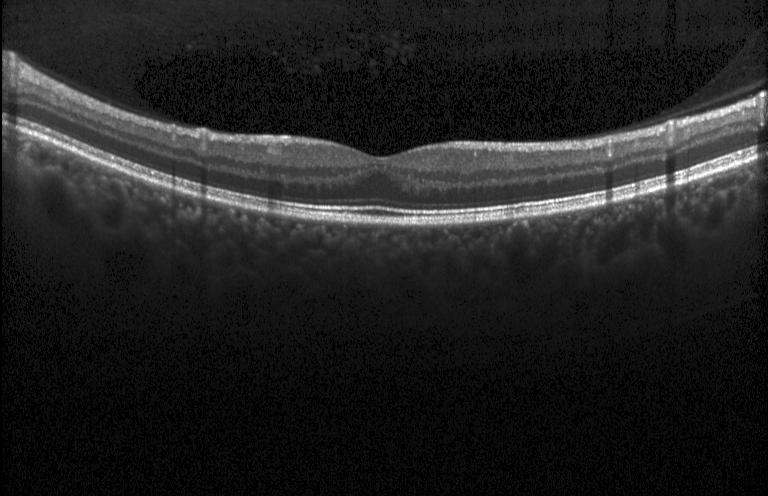

OCT line scan
No evidence of CNV, DME, or drusen.